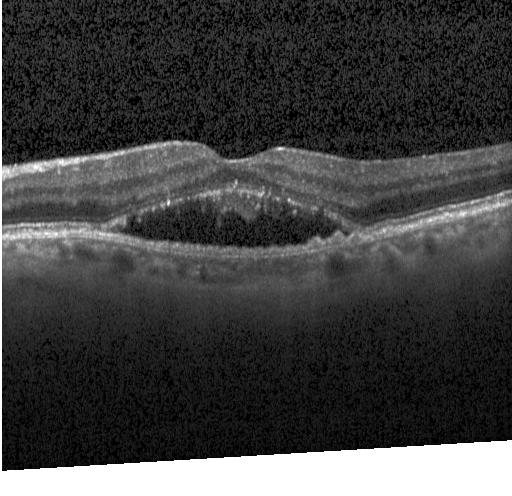
Macular OCT: choroidal neovascularization (CNV).